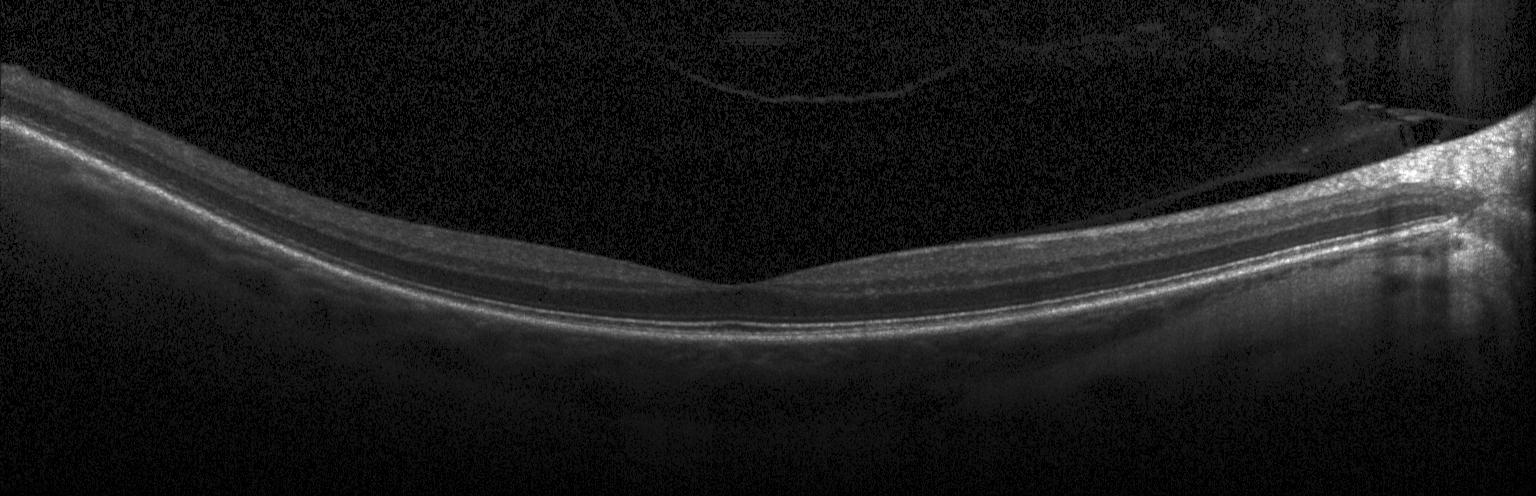 Retinal OCT B-scan.
Assessment: no CNV, no DME, and no drusen.